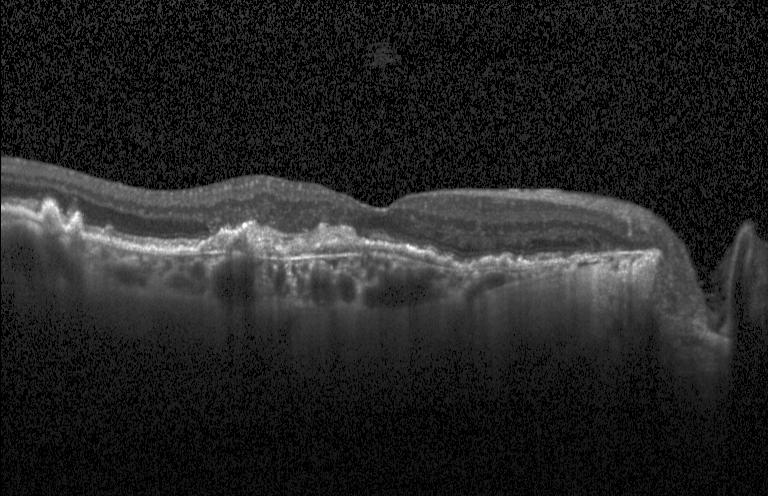 Optical coherence tomography B-scan. SD-OCT — A choroidal neovascular membrane.